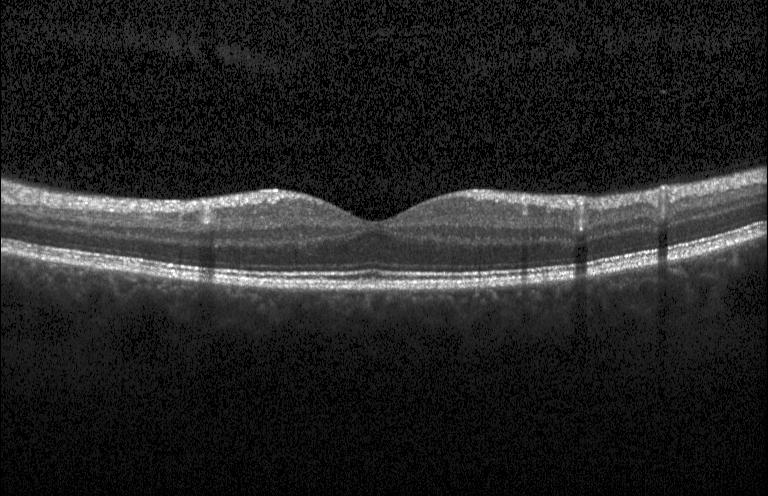
Spectral-domain OCT; instrument: Heidelberg Spectralis; optical coherence tomography B-scan; fovea-centered — Macular OCT: no choroidal neovascularization, no diabetic macular edema, and no drusen.